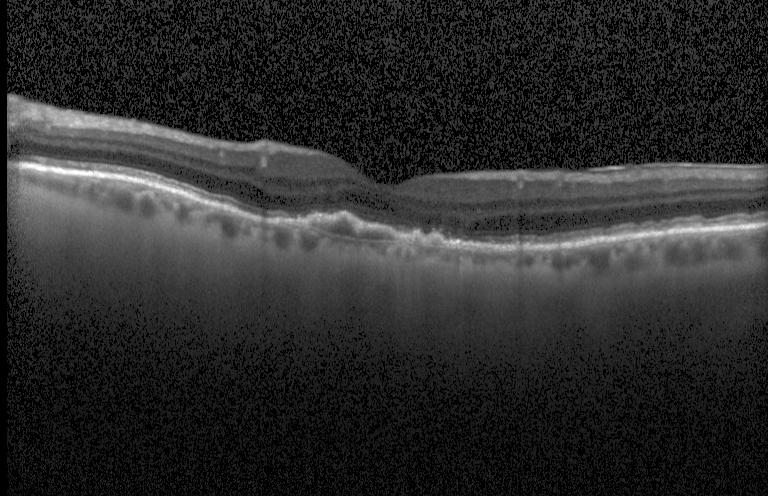 A choroidal neovascular membrane.